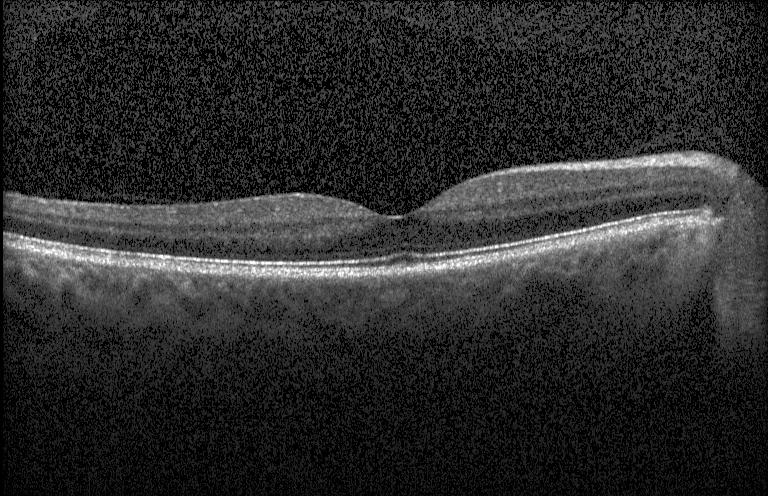
Acquired on a Heidelberg Spectralis, optical coherence tomography scan — Dx: no evidence of choroidal neovascularization, diabetic macular edema, or drusen.